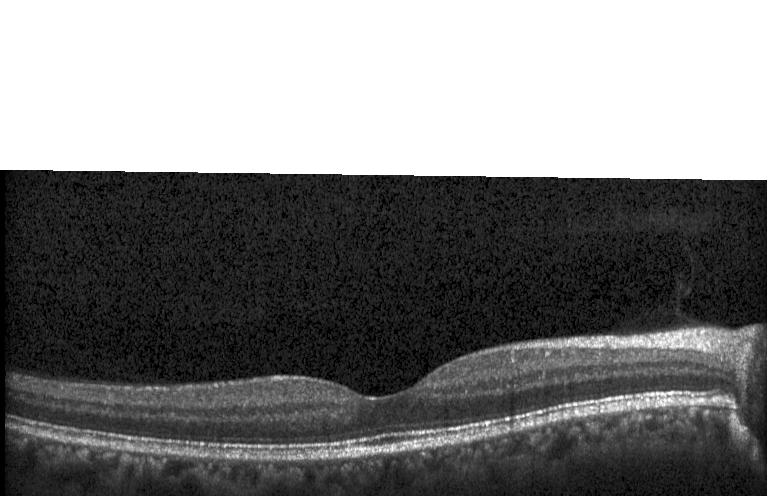
SD-OCT. Horizontal scan through the fovea. Optical coherence tomography B-scan. Heidelberg Spectralis OCT system. Diagnosis: no choroidal neovascularization, diabetic macular edema, or drusen.